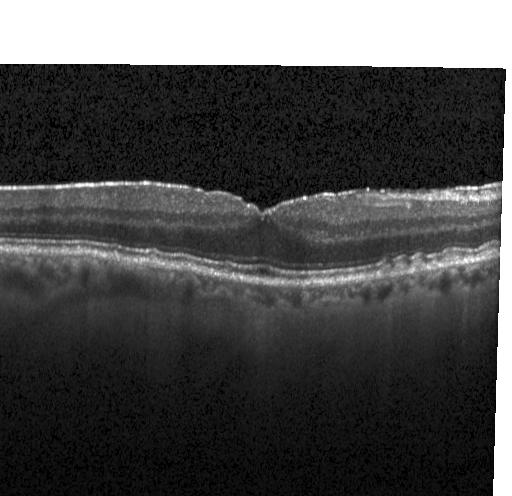
Dx: drusen.